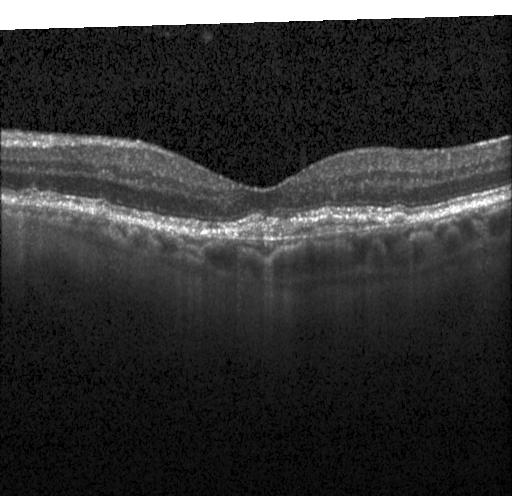
OCT line scan, through the macula
Choroidal neovascularization (CNV).